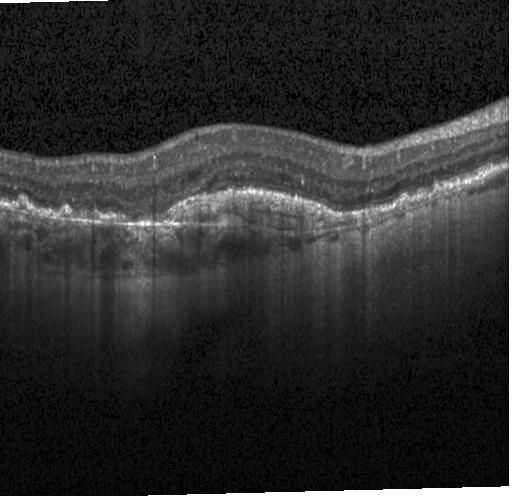 Spectral-domain optical coherence tomography · fovea-centered · instrument: Heidelberg Spectralis · retinal OCT cross-section.
Diagnosis: a choroidal neovascular membrane.